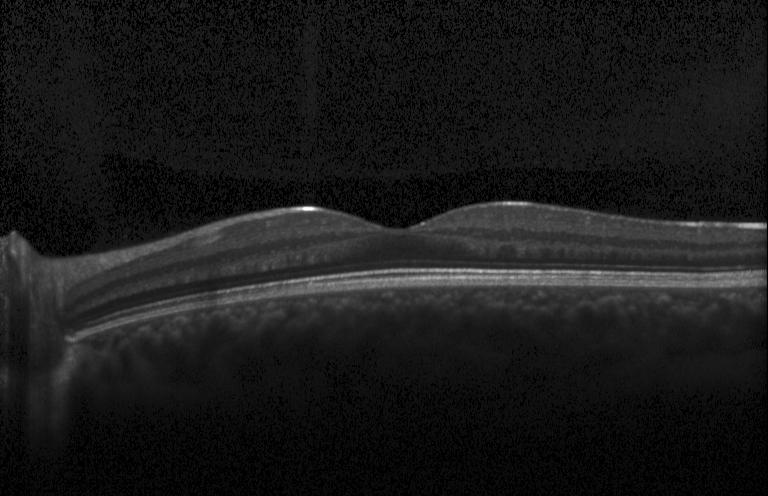

Spectral-domain OCT B-scan: no choroidal neovascularization, no diabetic macular edema, and no drusen.